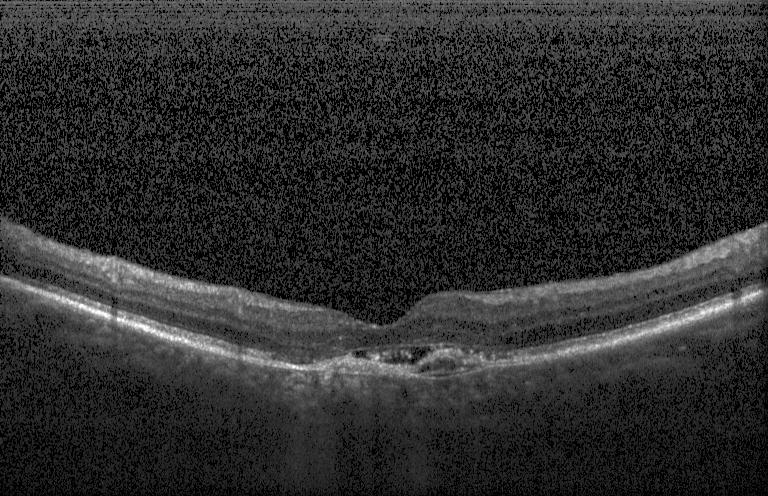 Retinal OCT cross-section showing a choroidal neovascular membrane.